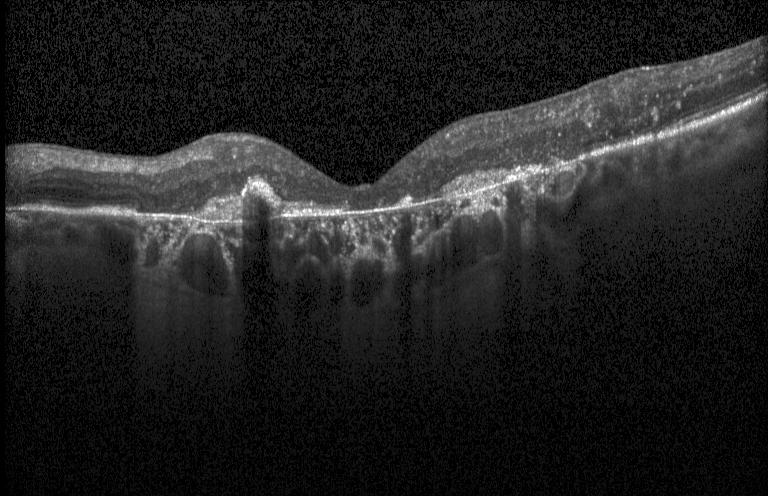

Impression: a choroidal neovascular membrane.